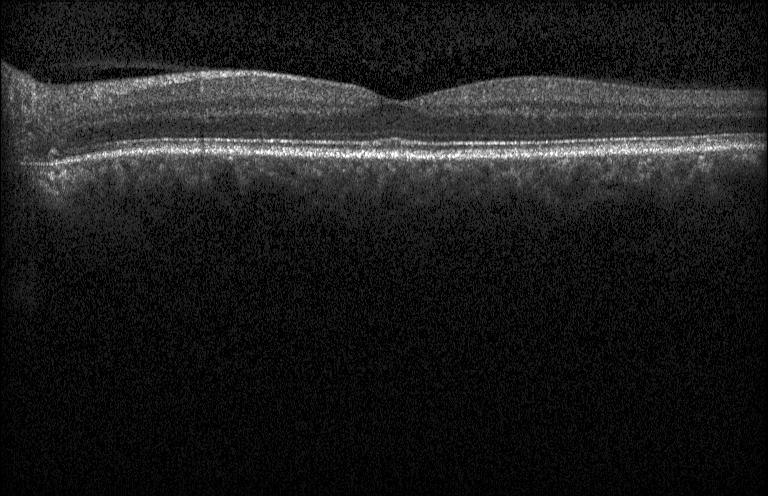 Diagnosis: no choroidal neovascularization, diabetic macular edema, or drusen.